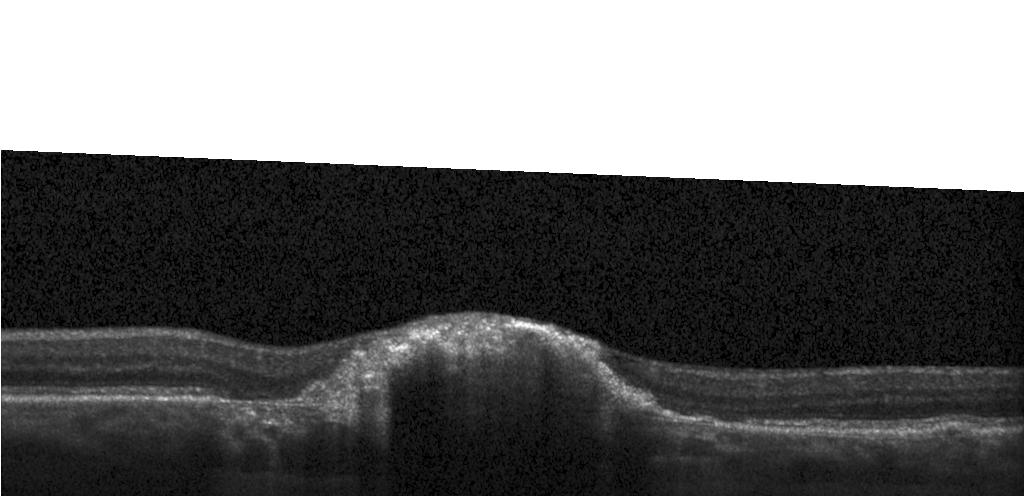
Optical coherence tomography B-scan, SD-OCT — Finding: a choroidal neovascular membrane.